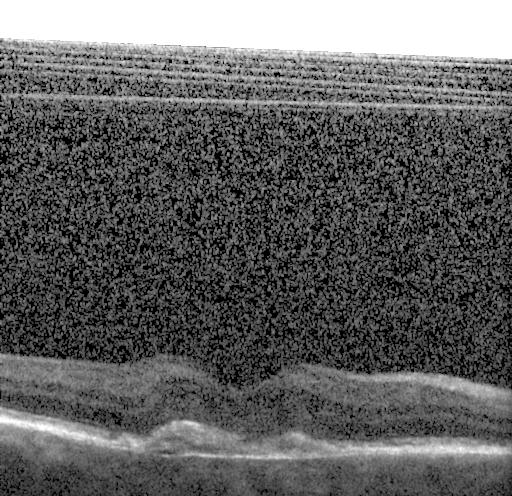 SD-OCT, Heidelberg Spectralis, optical coherence tomography B-scan, macular scan — Finding: CNV.